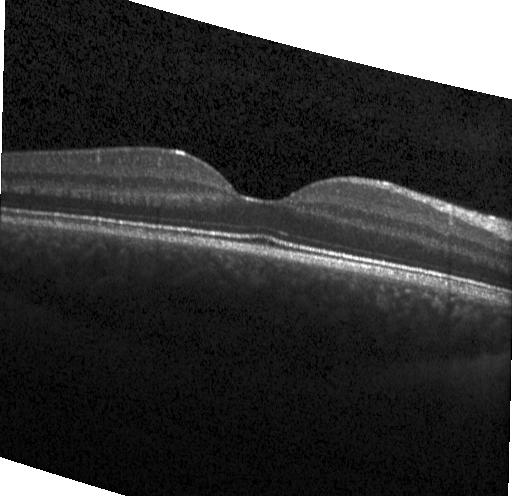 OCT B-scan.
Macular OCT: no choroidal neovascularization, no diabetic macular edema, and no drusen.